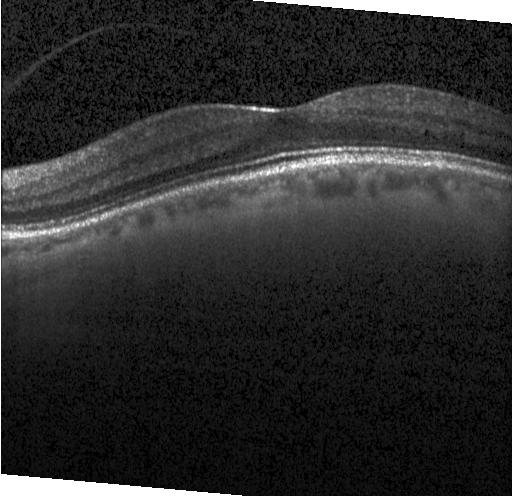

Instrument: Heidelberg Spectralis, spectral-domain OCT, OCT B-scan, fovea-centered
Impression: neither choroidal neovascularization, diabetic macular edema, nor drusen.